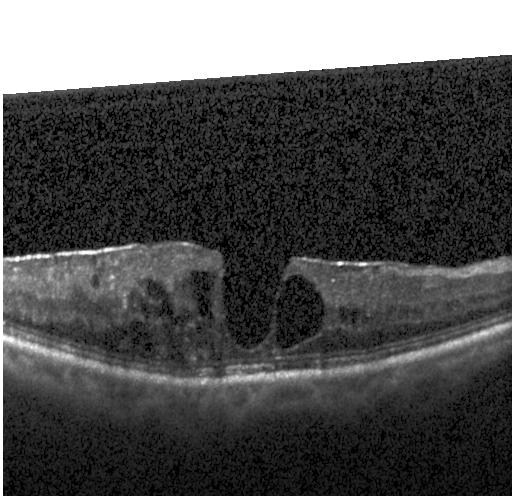
Diagnosis: diabetic macular edema.